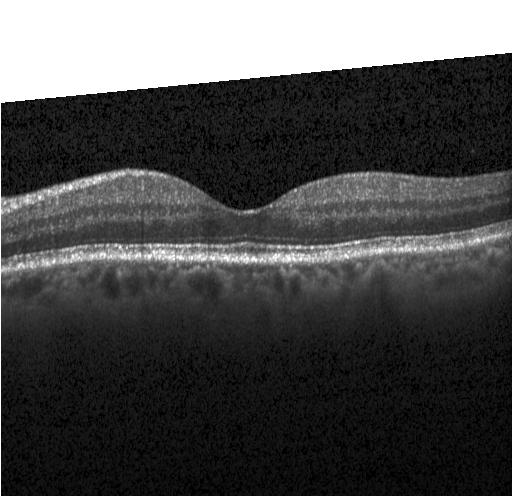 Optical coherence tomography scan · spectral-domain OCT.
Assessment: no CNV, no DME, and no drusen.